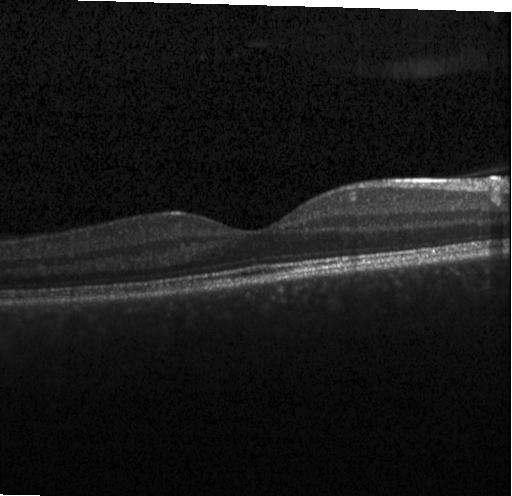 Optical coherence tomography B-scan. Spectral-domain OCT.
Neither CNV, DME, nor drusen.